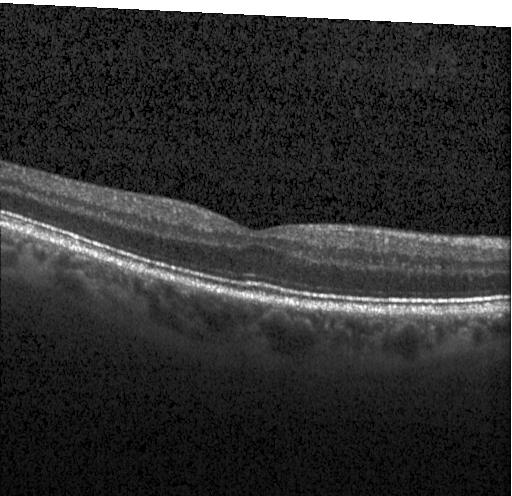

Instrument: Heidelberg Spectralis, optical coherence tomography B-scan
Finding: no evidence of choroidal neovascularization, diabetic macular edema, or drusen.